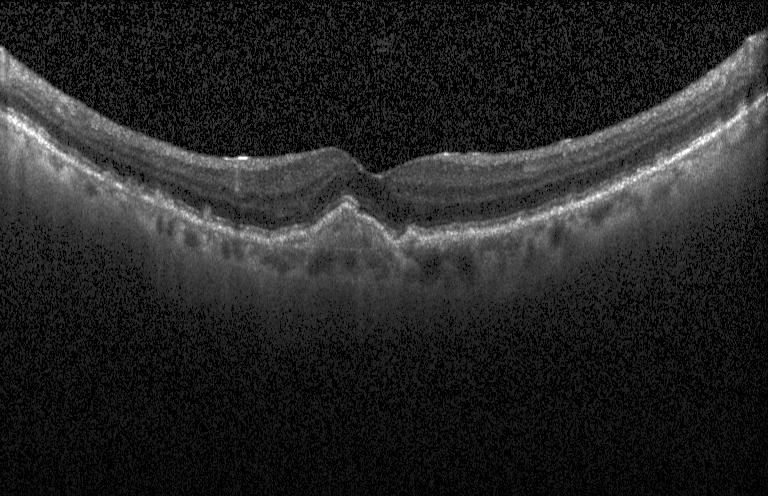

Heidelberg Spectralis; spectral-domain OCT; retinal OCT B-scan.
Impression: a choroidal neovascular membrane.